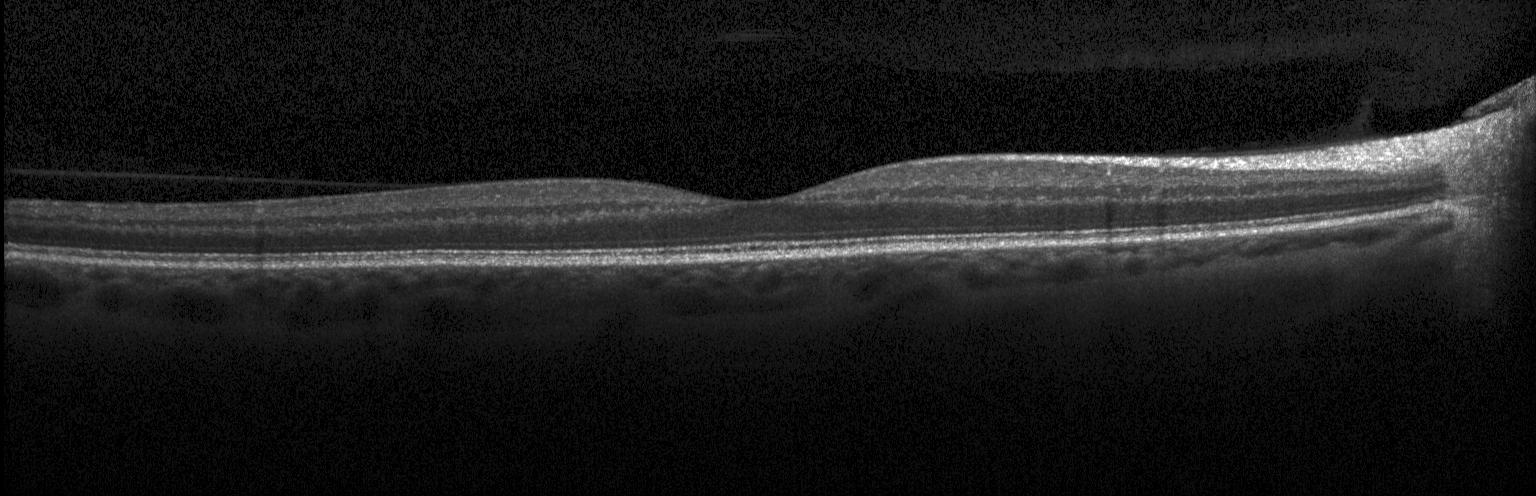

Optical coherence tomography B-scan; instrument: Heidelberg Spectralis
Impression: no choroidal neovascularization, no diabetic macular edema, and no drusen.